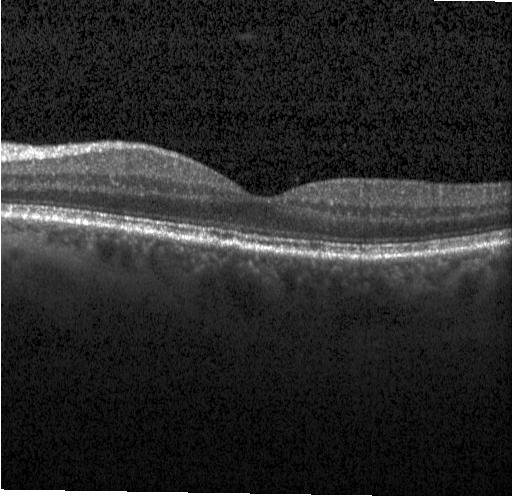 Diagnosis: no choroidal neovascularization, diabetic macular edema, or drusen.